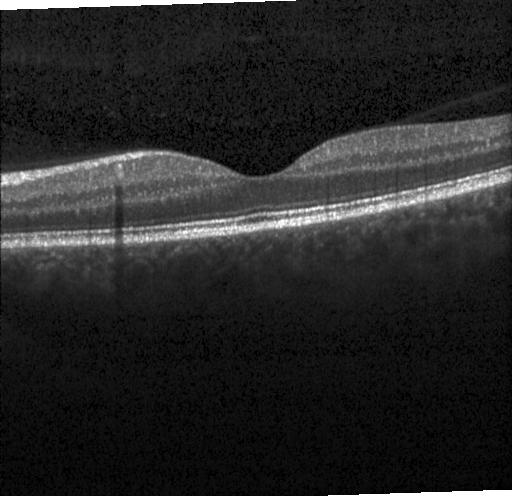 Optical coherence tomography scan; spectral-domain optical coherence tomography; Heidelberg Spectralis. The scan shows no evidence of CNV, DME, or drusen.